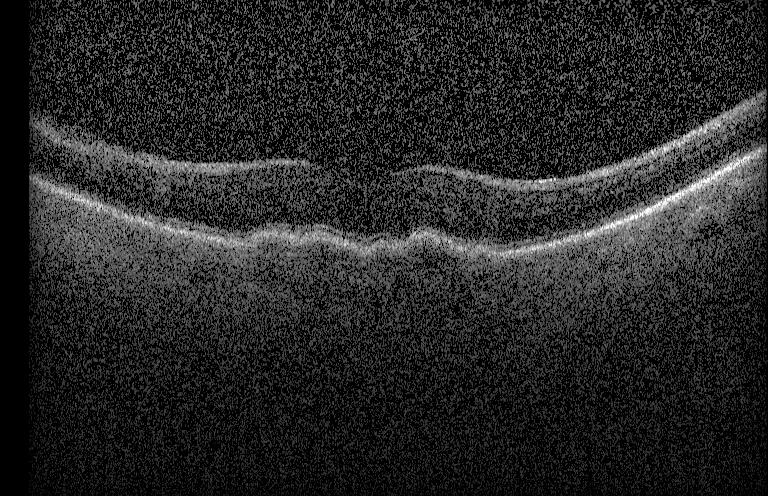

OCT line scan · Heidelberg Spectralis · spectral-domain OCT · macular scan — Diagnosis: choroidal neovascularization.